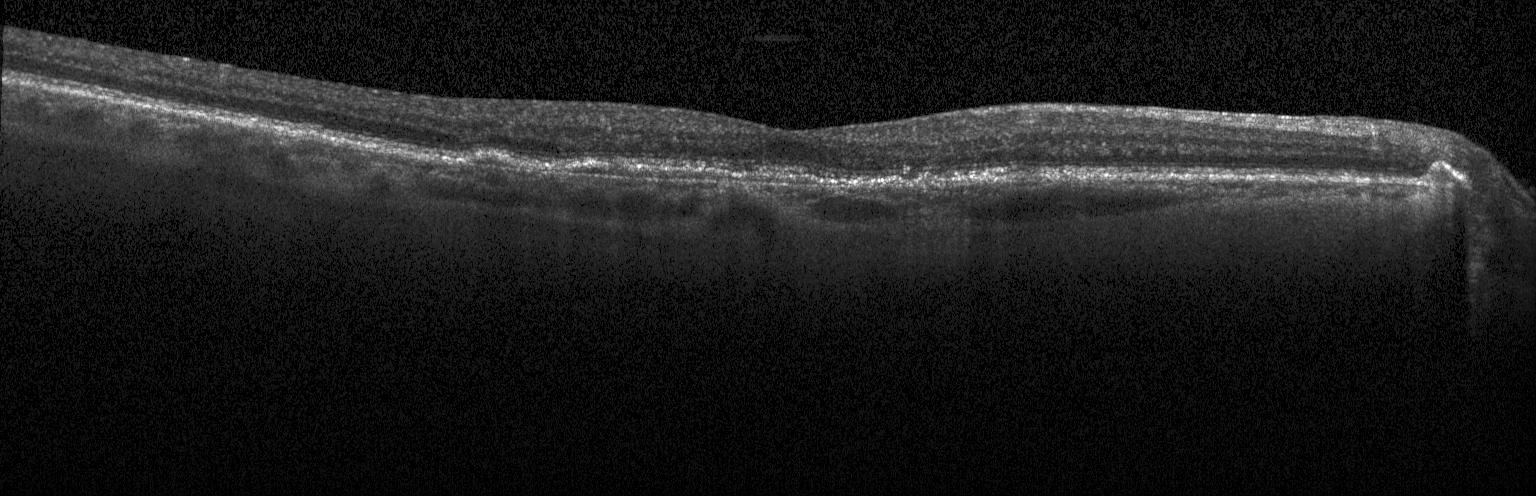

Heidelberg Spectralis, retinal OCT B-scan, spectral-domain optical coherence tomography
Impression: CNV.